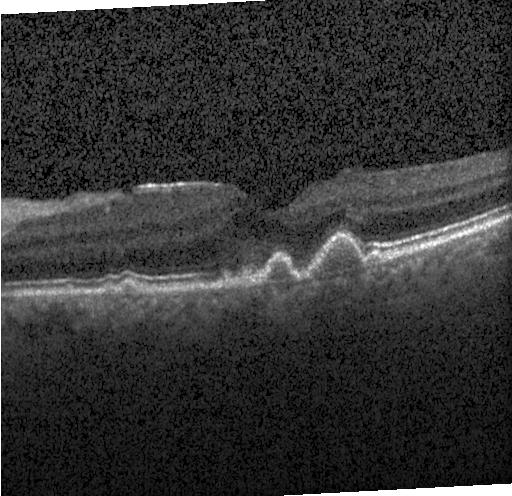
OCT B-scan. Macular scan. Acquired on a Heidelberg Spectralis.
Impression: sub-RPE drusenoid deposits.